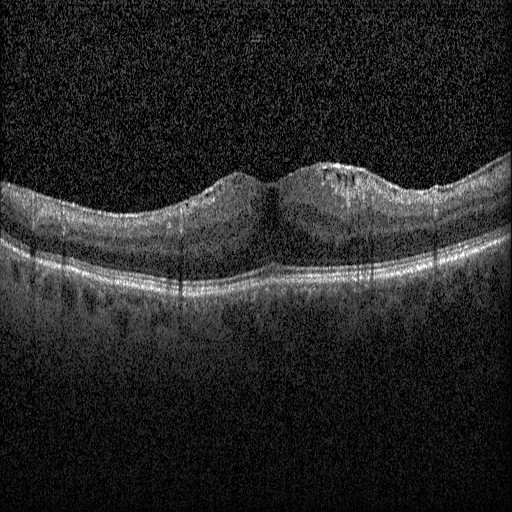
OCT line scan · acquired on a Heidelberg Spectralis
The scan shows DME.